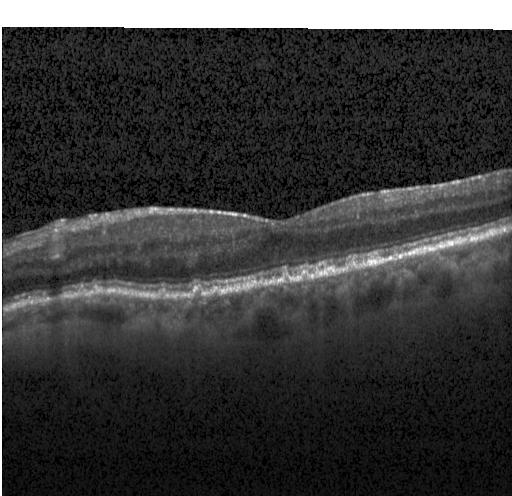
Optical coherence tomography B-scan · spectral-domain OCT — Finding: sub-RPE drusenoid deposits.